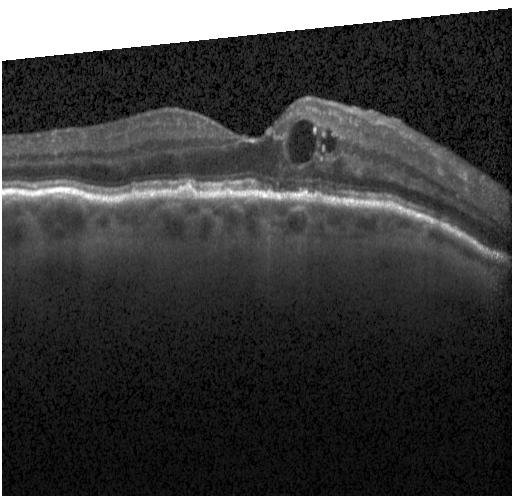 OCT B-scan showing choroidal neovascularization.